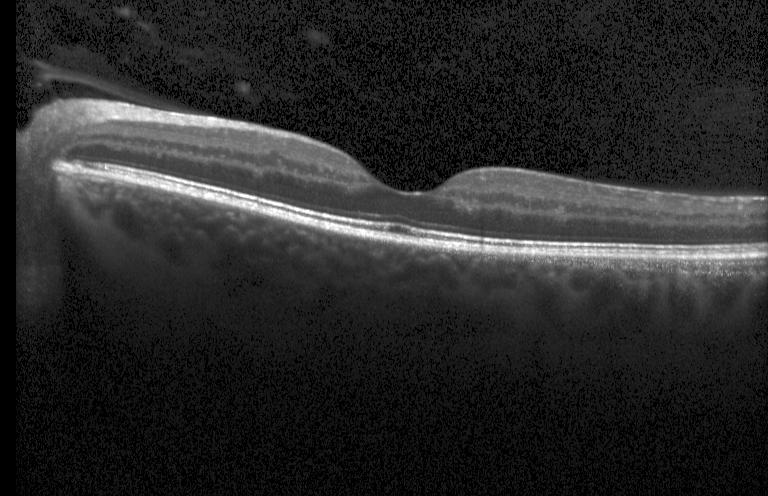
Optical coherence tomography B-scan — OCT finding: neither CNV, DME, nor drusen.